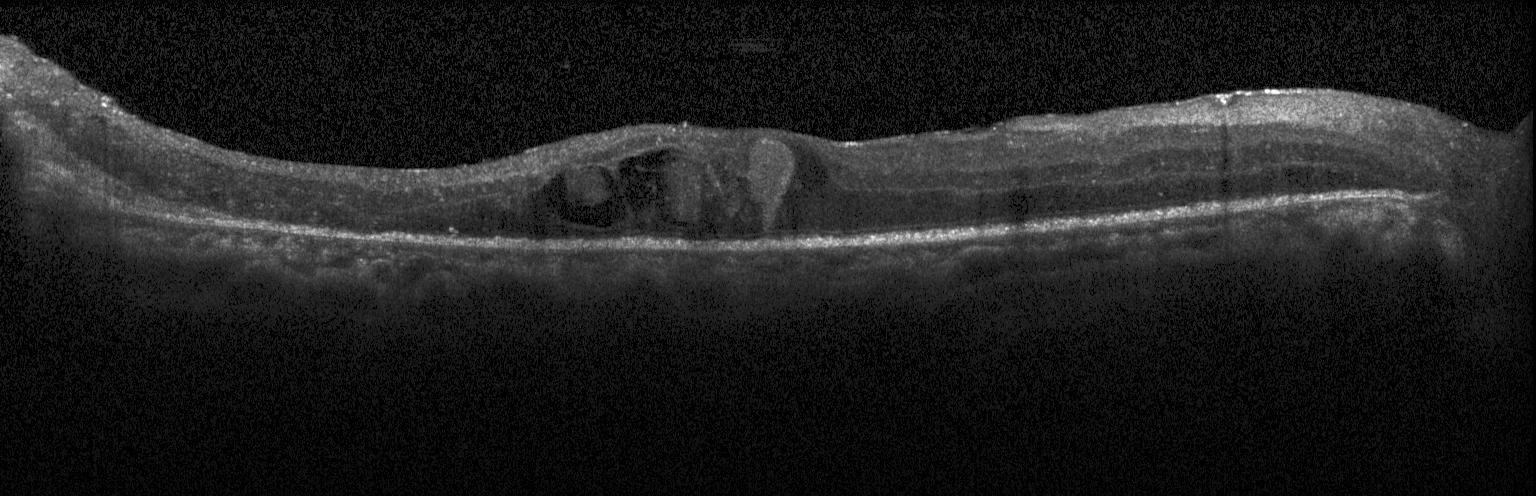 Retinal OCT cross-section; instrument: Heidelberg Spectralis
Finding: diabetic macular edema (DME).